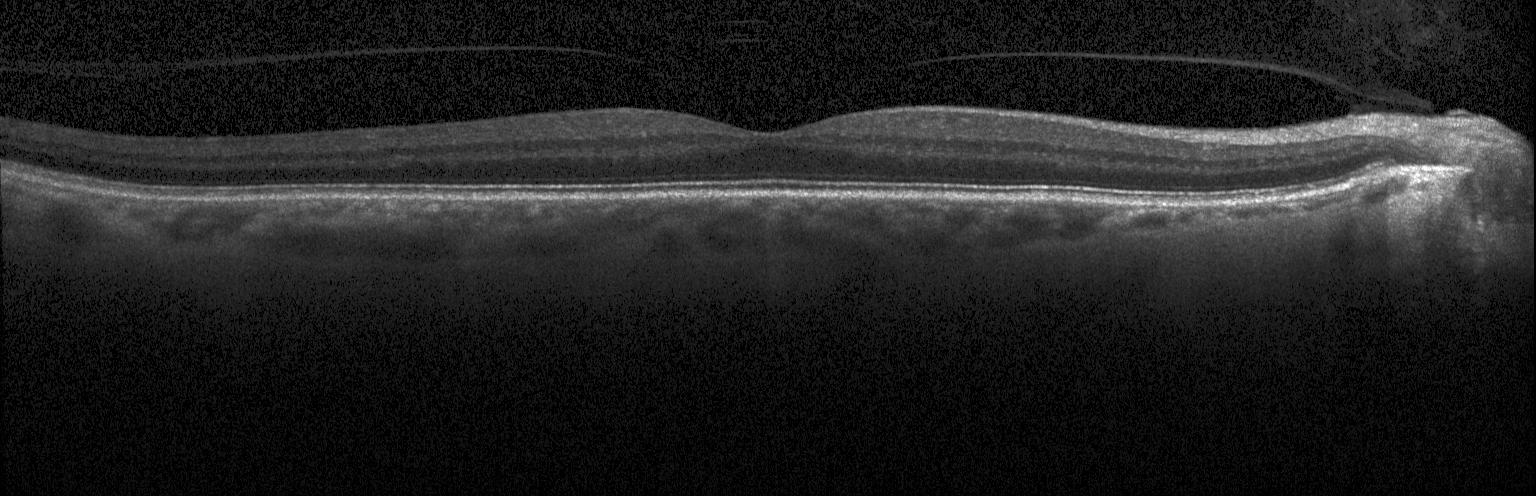

Spectral-domain optical coherence tomography. Optical coherence tomography scan.
Diagnosis: no choroidal neovascularization, no diabetic macular edema, and no drusen.